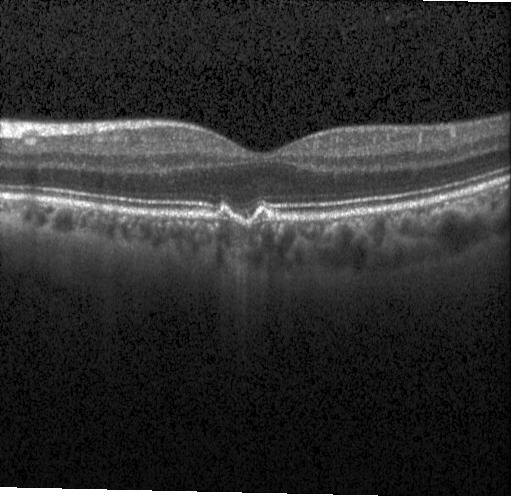
Assessment: sub-RPE drusenoid deposits.